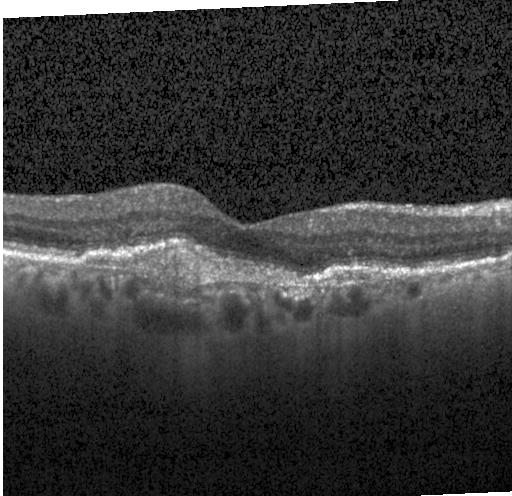

Finding: a choroidal neovascular membrane.